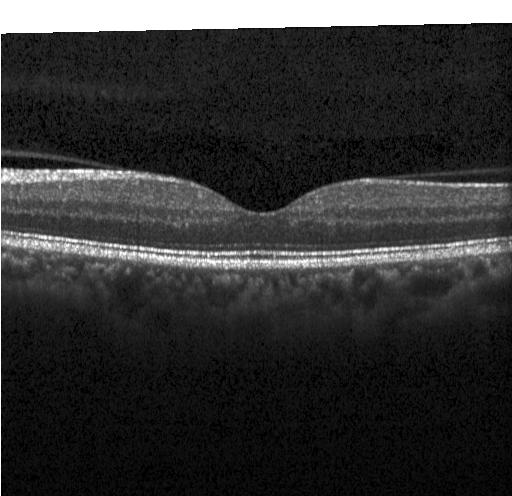
Impression: no evidence of choroidal neovascularization, diabetic macular edema, or drusen.